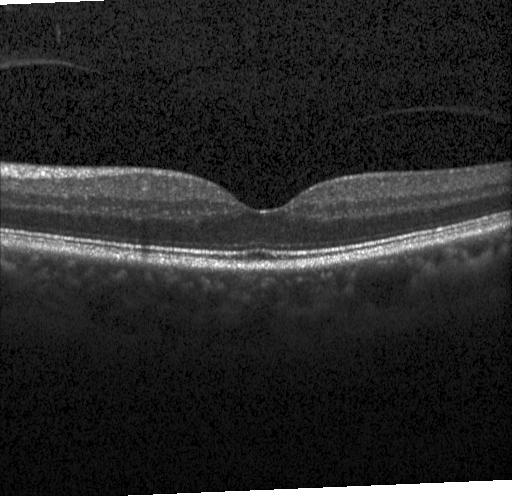
Optical coherence tomography B-scan — The scan shows no choroidal neovascularization, diabetic macular edema, or drusen.